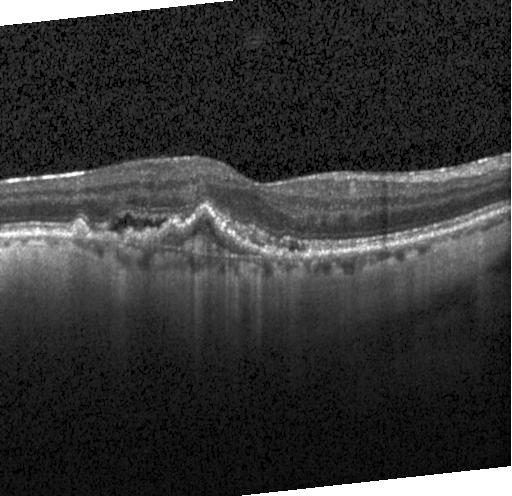

Macular scan; retinal OCT B-scan; SD-OCT — Impression: CNV.